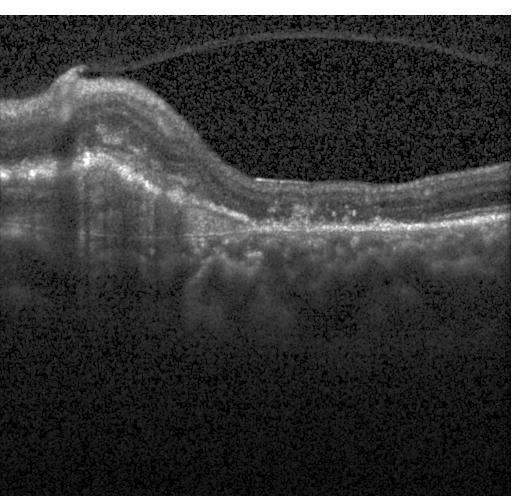 Optical coherence tomography B-scan
Macular OCT: choroidal neovascularization.